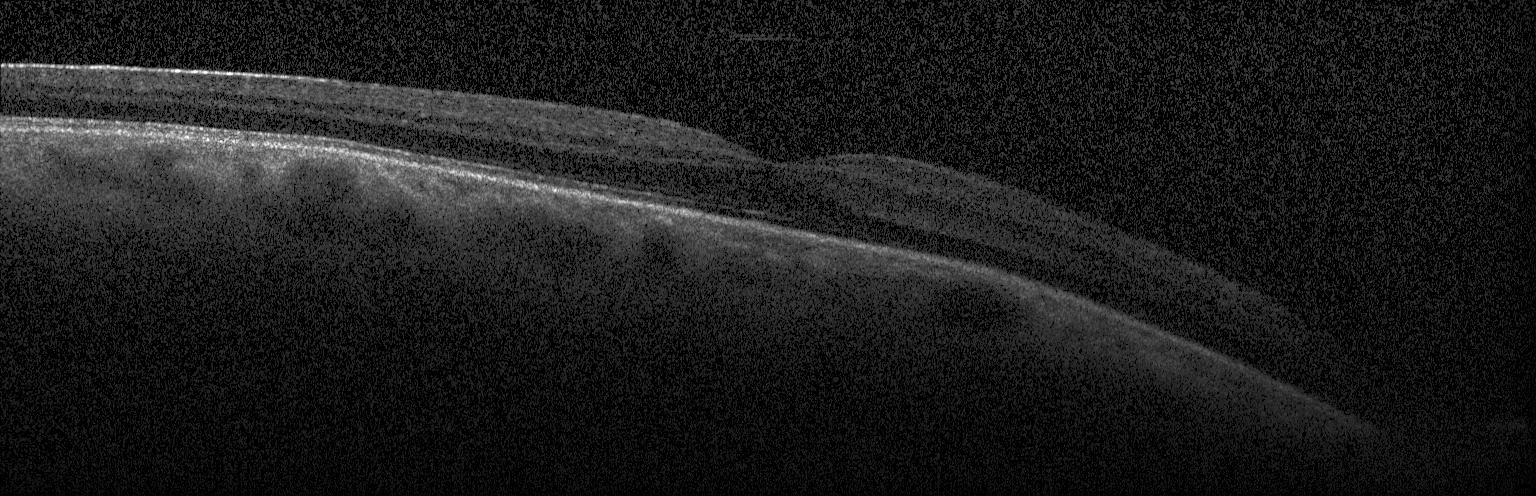

Retinal OCT B-scan — The scan shows no evidence of choroidal neovascularization, diabetic macular edema, or drusen.